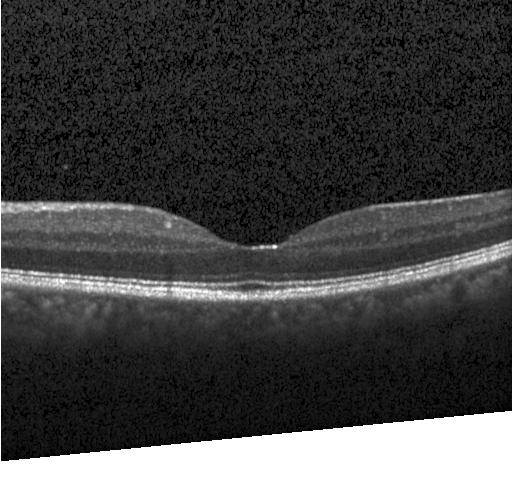 Impression: neither choroidal neovascularization, diabetic macular edema, nor drusen.